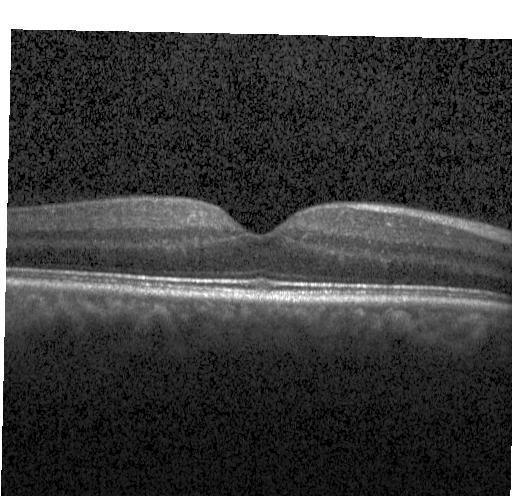

SD-OCT; acquired on a Heidelberg Spectralis; OCT line scan.
Finding: no evidence of choroidal neovascularization, diabetic macular edema, or drusen.